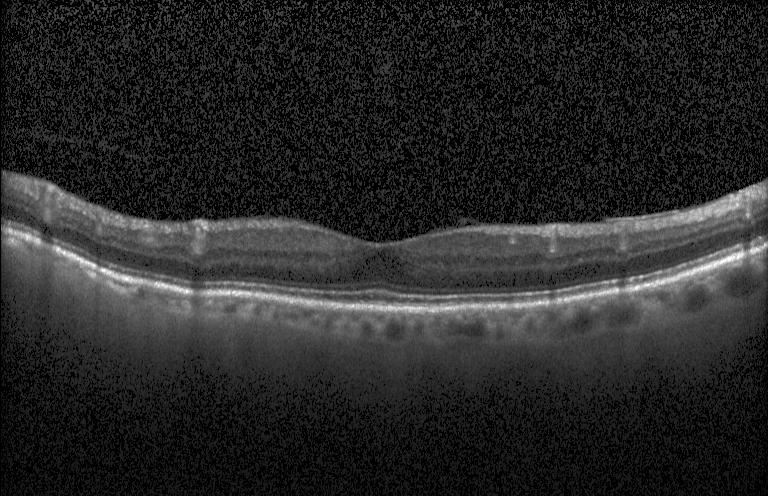

Horizontal scan through the fovea, retinal OCT B-scan
Dx: neither CNV, DME, nor drusen.